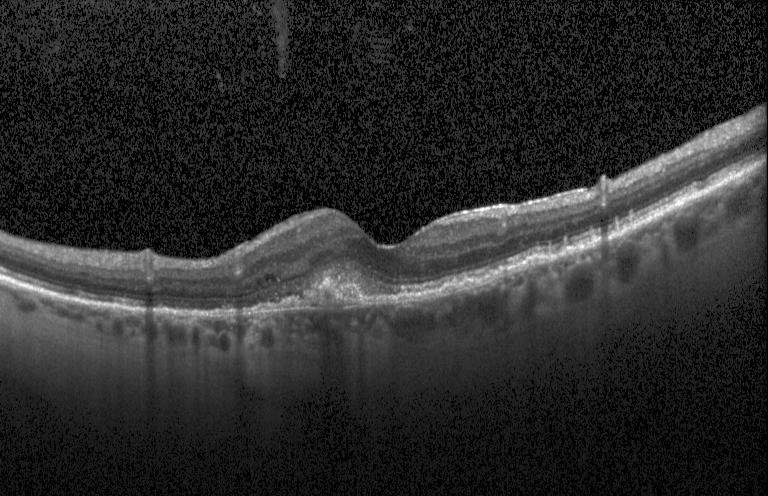 Diagnosis: a choroidal neovascular membrane.